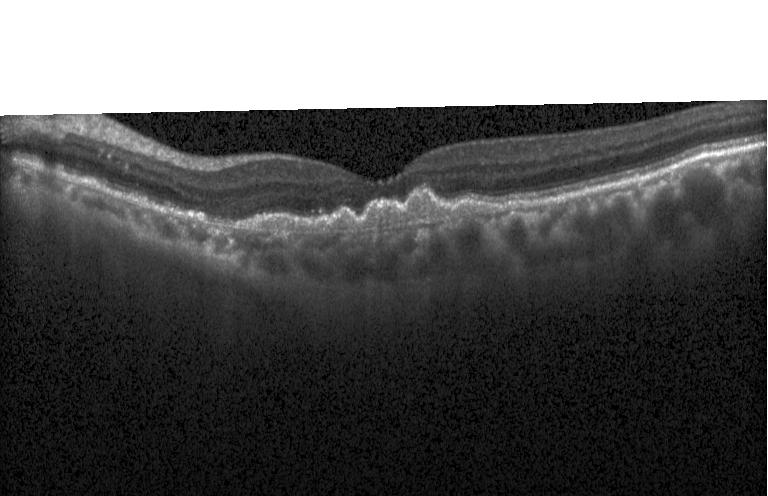
Dx: a choroidal neovascular membrane.